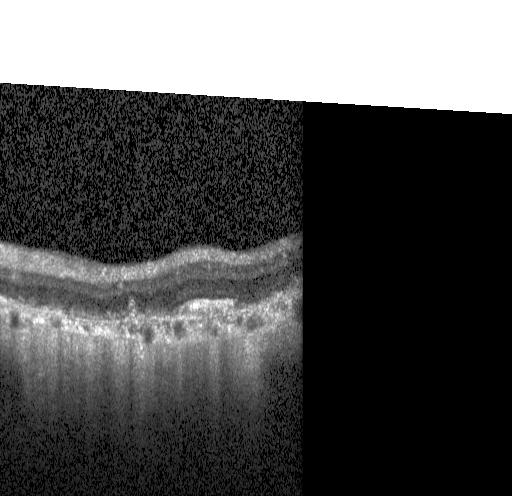
OCT line scan
Impression: choroidal neovascularization.